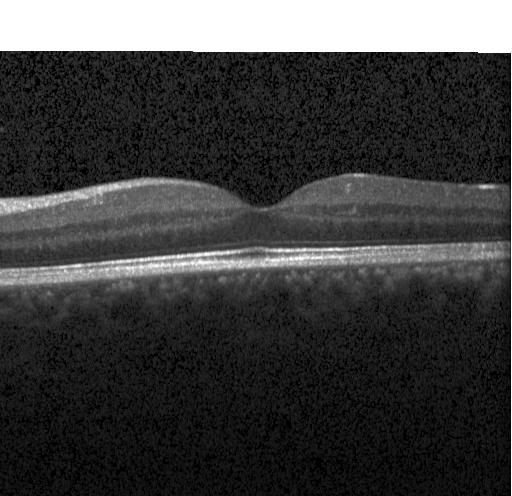

Acquired on a Heidelberg Spectralis; OCT line scan; SD-OCT.
Assessment: no choroidal neovascularization, diabetic macular edema, or drusen.